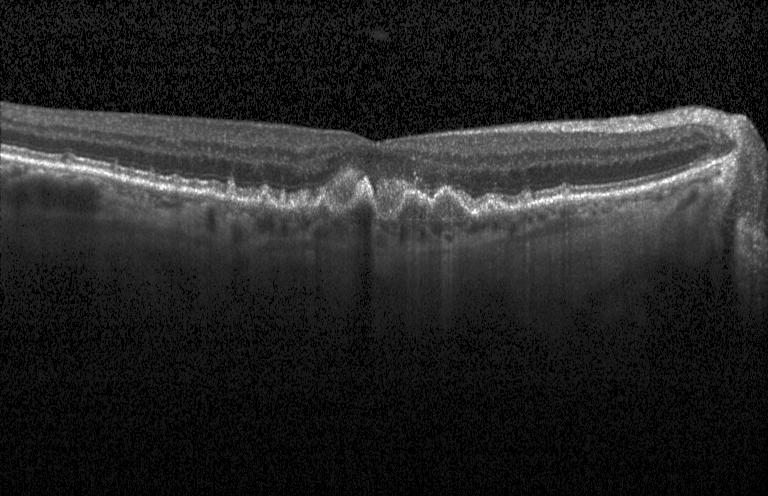
OCT B-scan. Heidelberg Spectralis OCT system — Diagnosis: choroidal neovascularization.